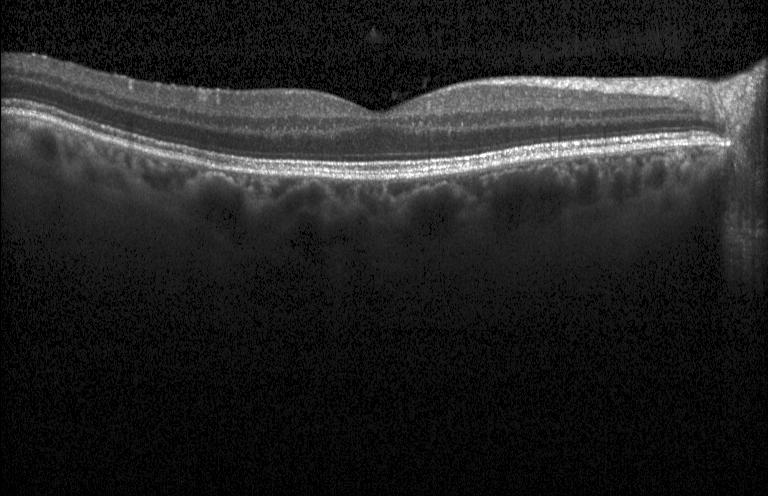

Instrument: Heidelberg Spectralis, OCT B-scan — Diagnosis: neither choroidal neovascularization, diabetic macular edema, nor drusen.